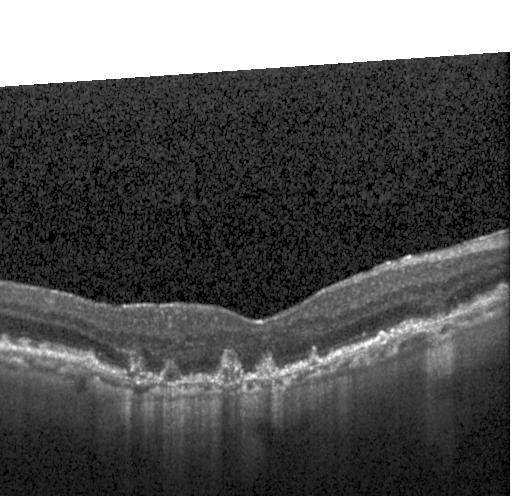
Through the macula, OCT B-scan.
Diagnosis: choroidal neovascularization (CNV).